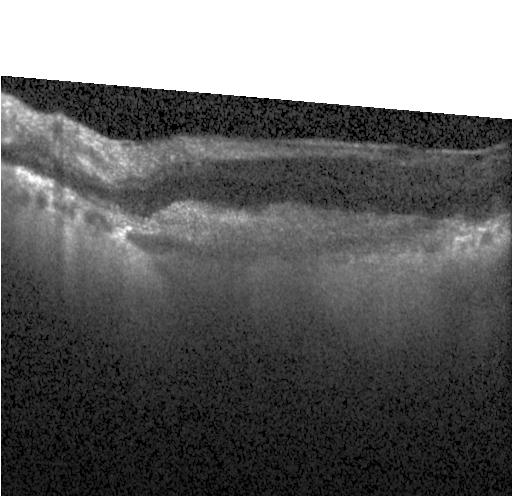

Macular scan; retinal OCT B-scan; spectral-domain OCT.
Choroidal neovascularization.